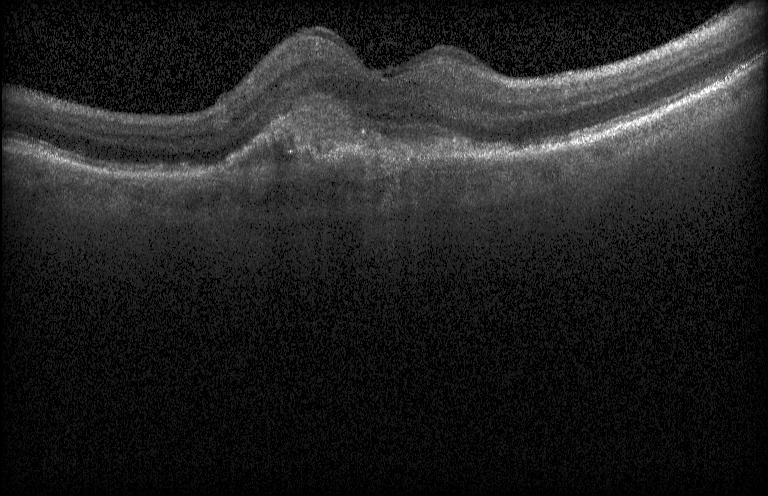
Retinal OCT B-scan. Acquired on a Heidelberg Spectralis. Diagnosis: choroidal neovascularization.